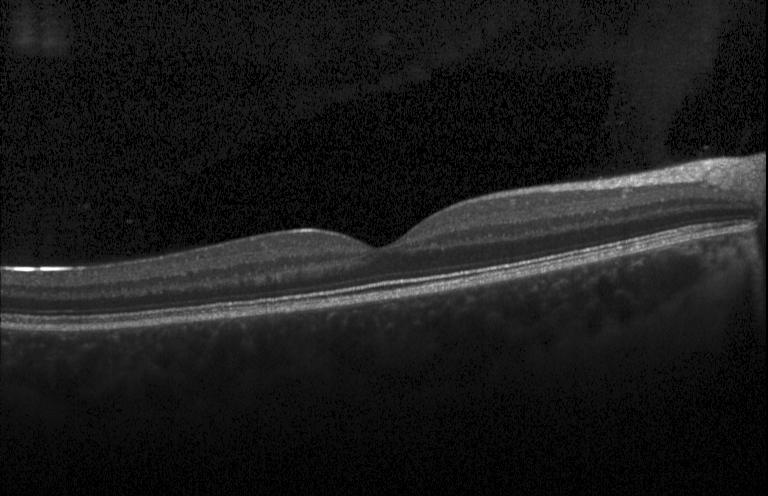
Optical coherence tomography B-scan; Heidelberg Spectralis OCT system; macular scan.
Finding: no CNV, DME, or drusen.